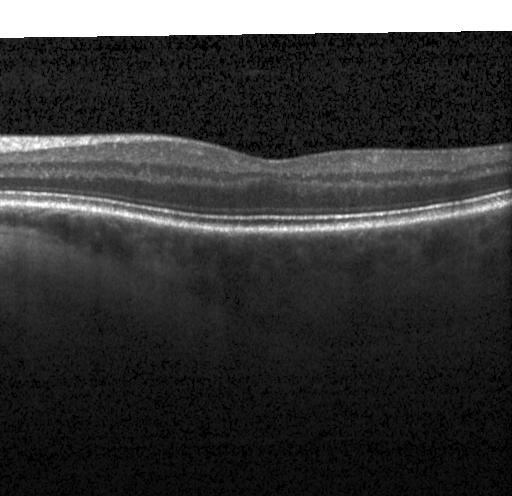

Retinal OCT B-scan
OCT finding: no CNV, DME, or drusen.